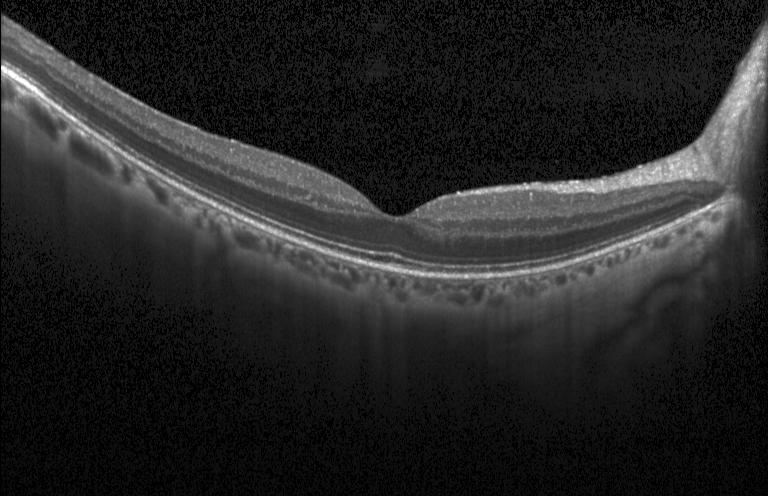

Finding: no choroidal neovascularization, diabetic macular edema, or drusen.